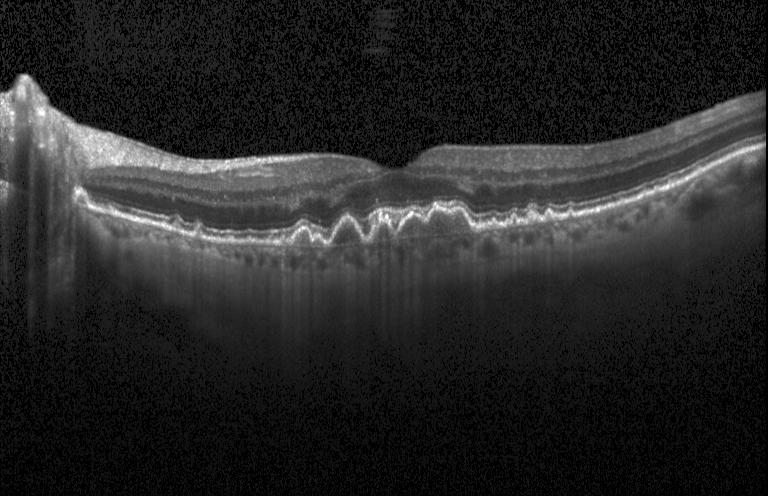 Dx: drusen.